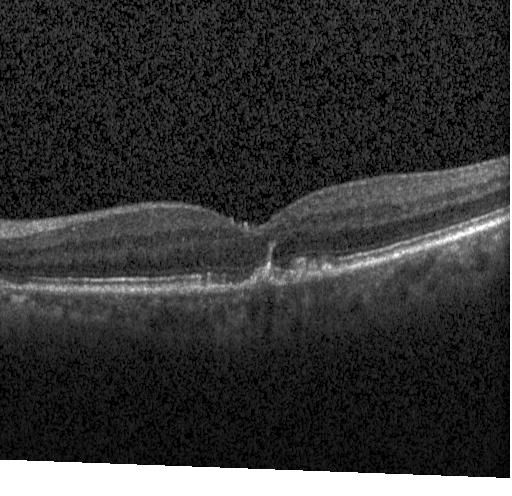

Retinal OCT cross-section, SD-OCT — Diagnosis: sub-RPE drusenoid deposits.